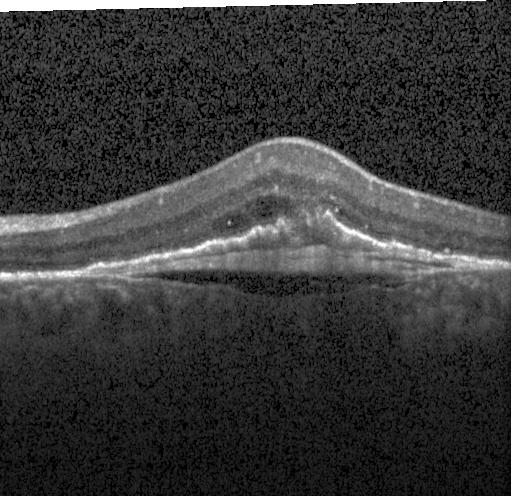 OCT B-scan showing CNV.